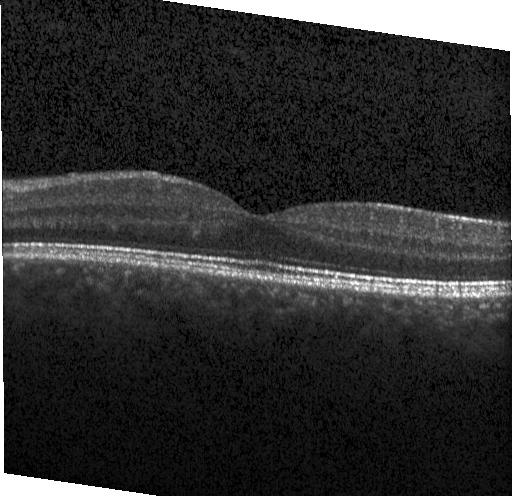
Macular OCT demonstrating neither choroidal neovascularization, diabetic macular edema, nor drusen.